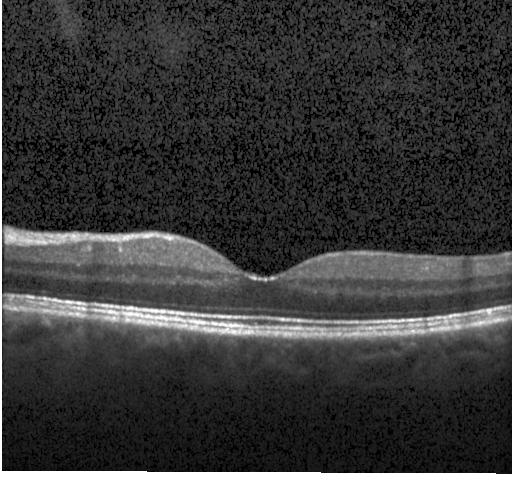
OCT finding: no CNV, no DME, and no drusen.